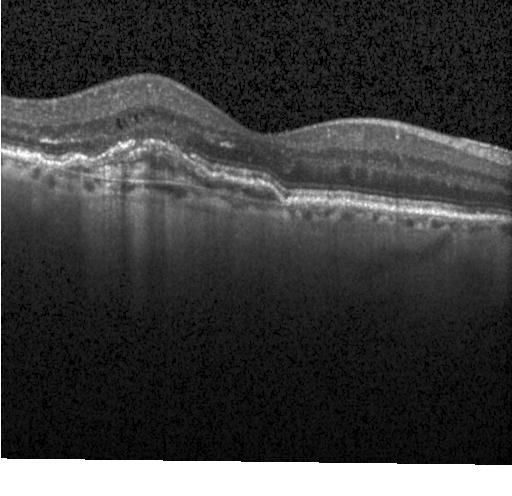

Retinal OCT cross-section. Acquired on a Heidelberg Spectralis. SD-OCT. Centered on the fovea. Finding: choroidal neovascularization (CNV).